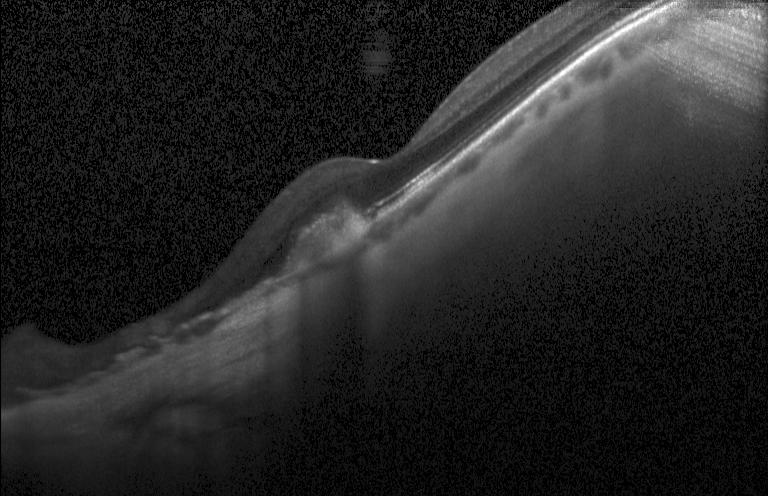
Heidelberg Spectralis. Horizontal scan through the fovea. Spectral-domain OCT. Optical coherence tomography B-scan
Impression: choroidal neovascularization (CNV).